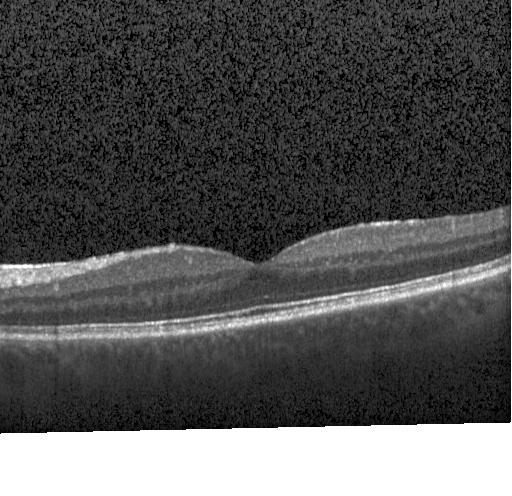

Spectral-domain optical coherence tomography · optical coherence tomography B-scan.
The scan shows no evidence of choroidal neovascularization, diabetic macular edema, or drusen.